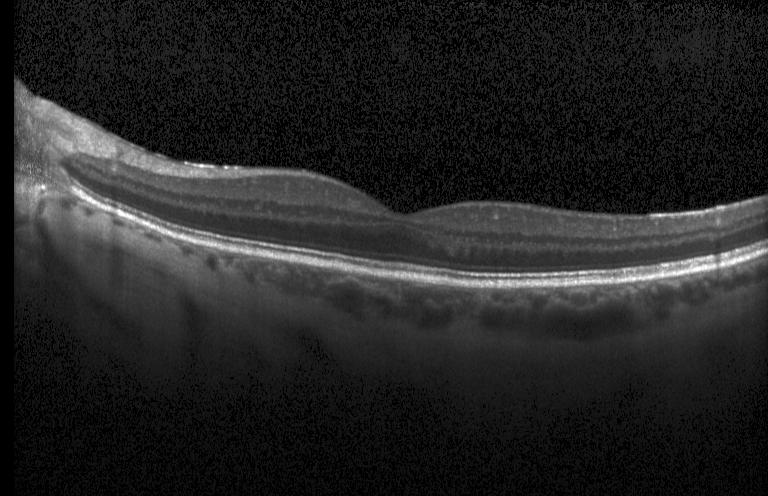
Assessment: no evidence of choroidal neovascularization, diabetic macular edema, or drusen.